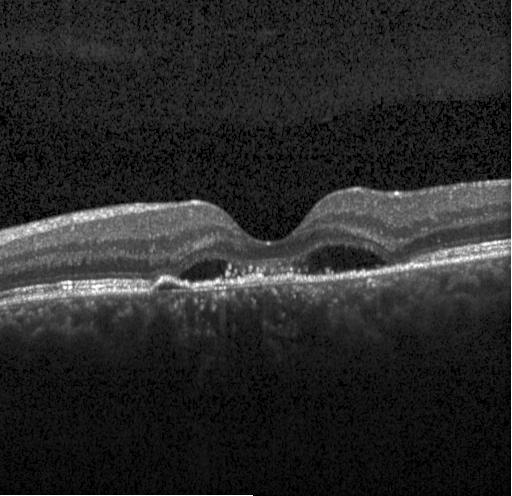

Horizontal scan through the fovea; retinal OCT B-scan.
OCT finding: choroidal neovascularization.